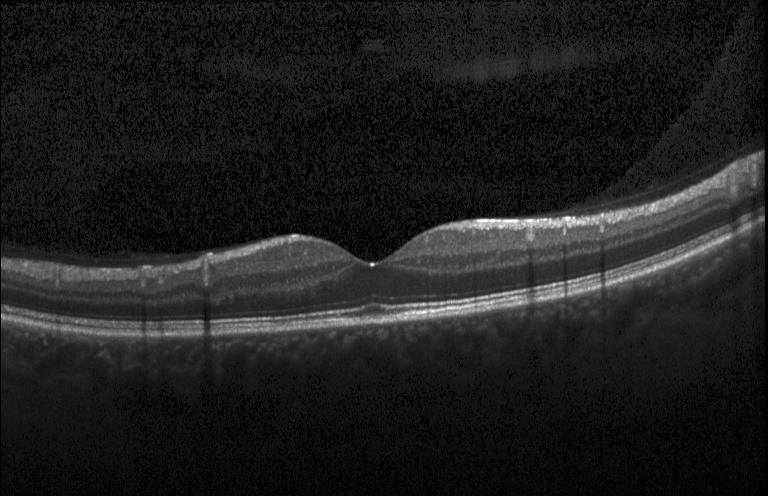 Macular OCT demonstrating neither choroidal neovascularization, diabetic macular edema, nor drusen.